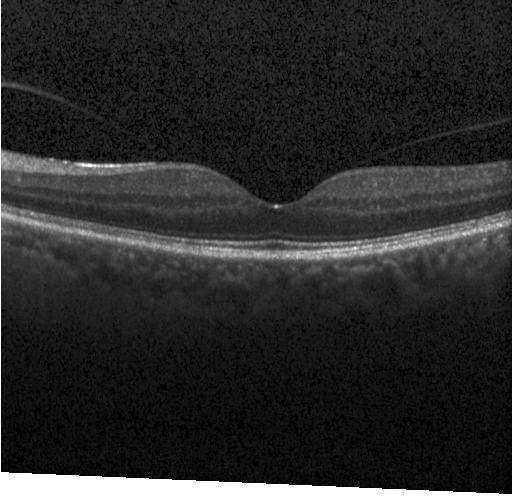
Diagnosis: neither CNV, DME, nor drusen.